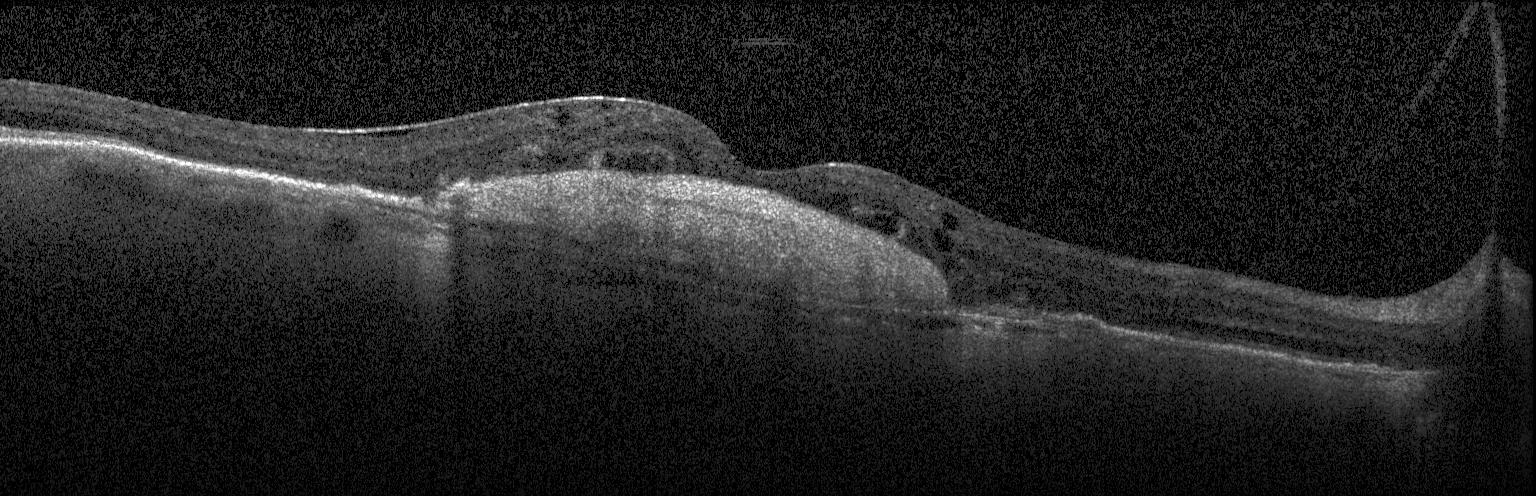
OCT scan showing a choroidal neovascular membrane.